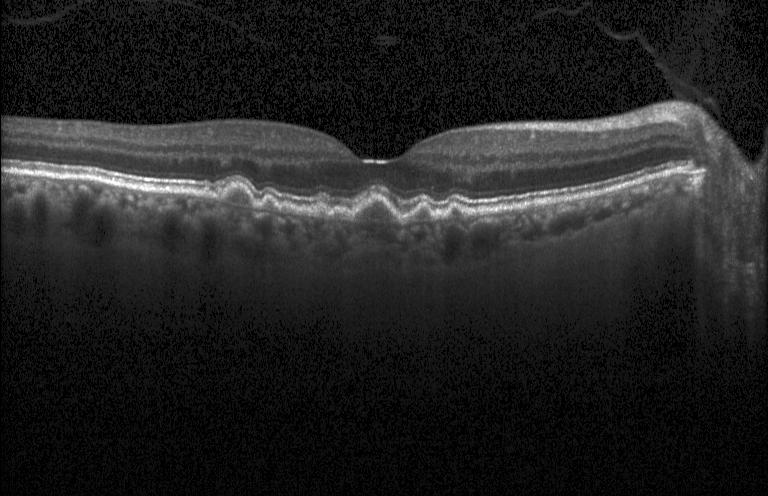

Optical coherence tomography scan — Diagnosis: multiple drusen.